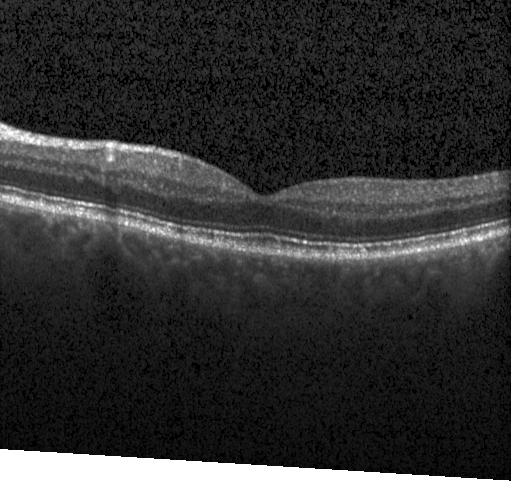
Diagnosis: neither CNV, DME, nor drusen.